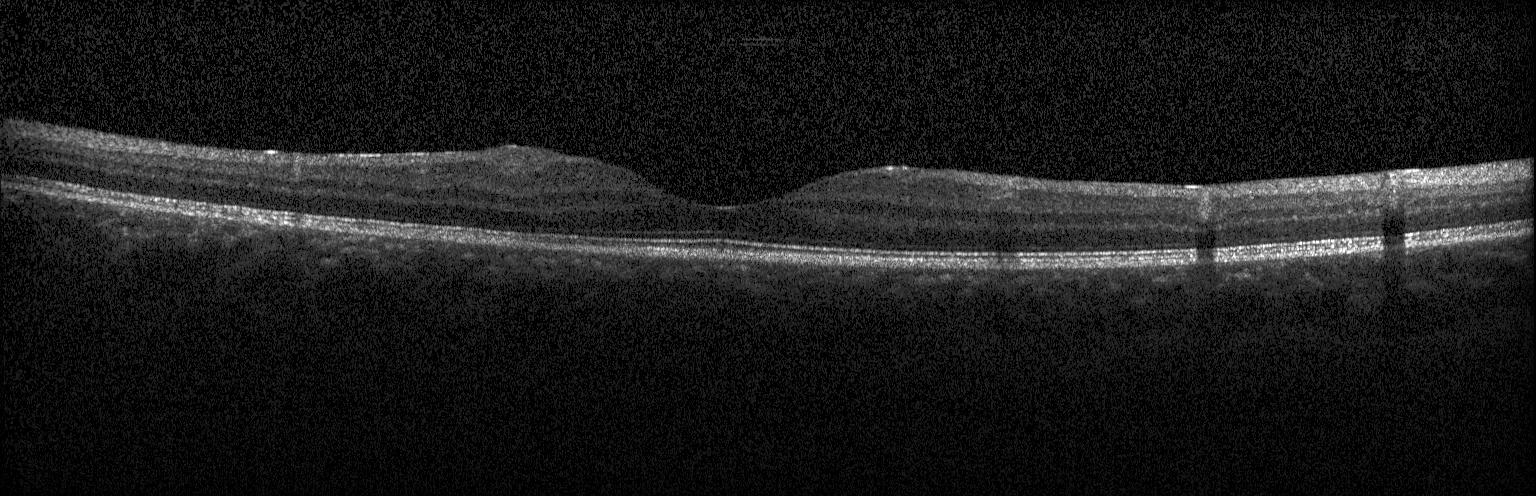
Finding: no choroidal neovascularization, no diabetic macular edema, and no drusen.